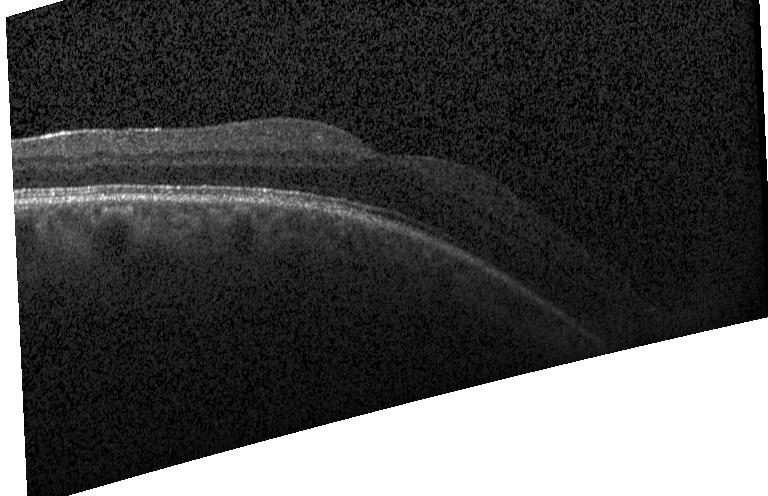 Heidelberg Spectralis OCT system. Spectral-domain optical coherence tomography. Optical coherence tomography scan
Finding: neither CNV, DME, nor drusen.